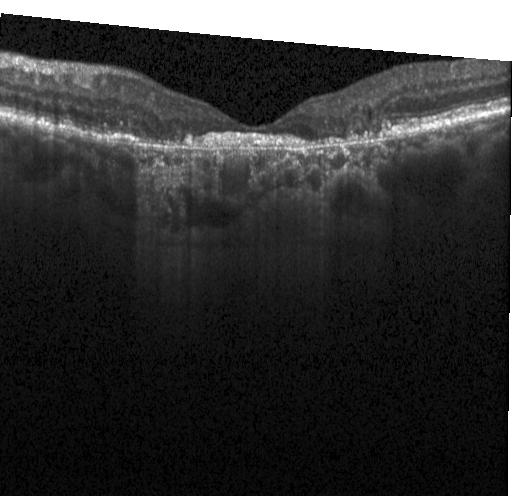
Retinal OCT B-scan — Assessment: a choroidal neovascular membrane.